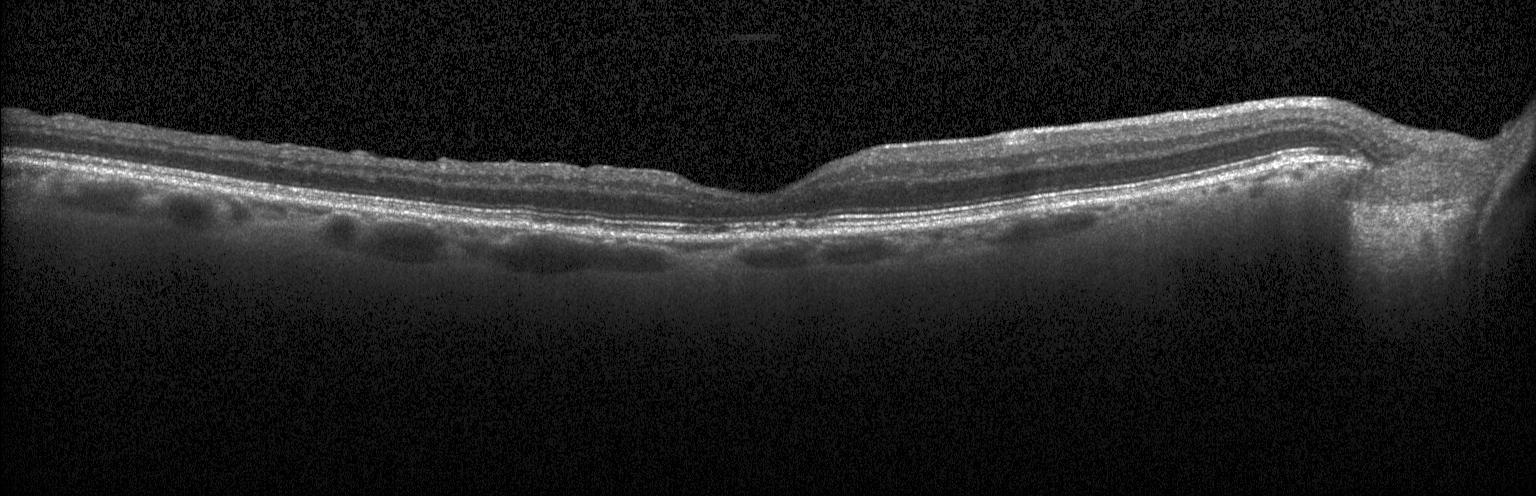 Heidelberg Spectralis · SD-OCT · OCT B-scan.
Finding: no choroidal neovascularization, diabetic macular edema, or drusen.